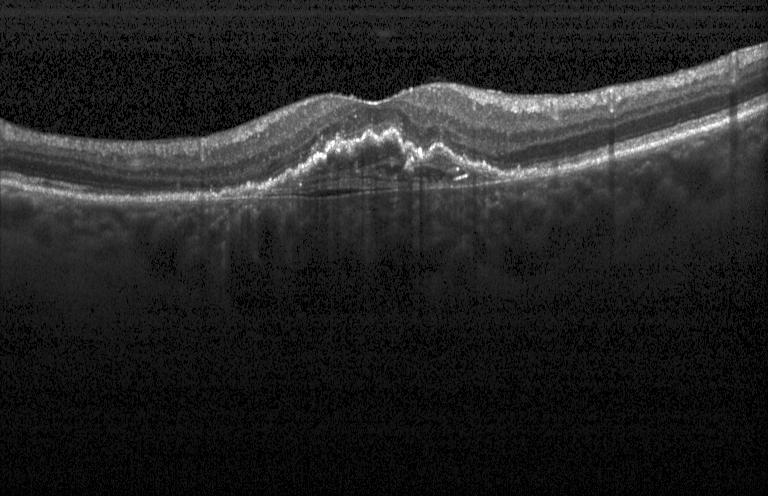
Acquired on a Heidelberg Spectralis. Macular scan. Optical coherence tomography B-scan — Choroidal neovascularization (CNV).